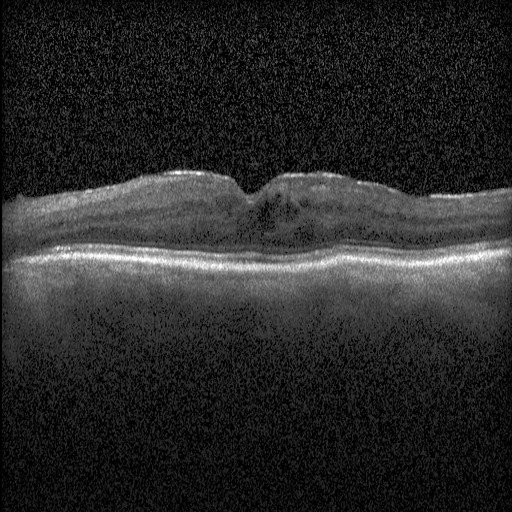

This B-scan demonstrates diabetic macular edema (DME).